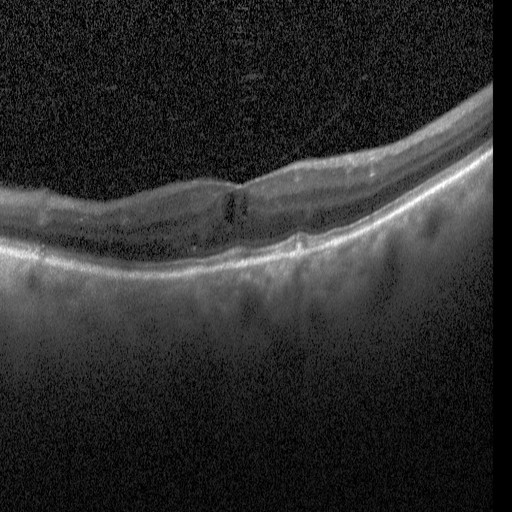

Instrument: Heidelberg Spectralis; spectral-domain OCT; macular scan; OCT line scan
Dx: diabetic macular edema.